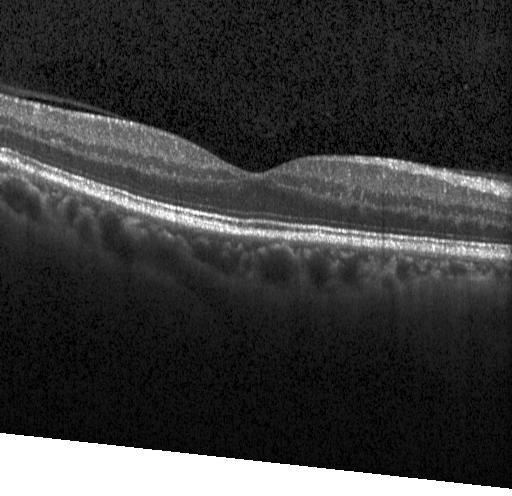
Horizontal scan through the fovea; Heidelberg Spectralis; OCT line scan
Impression: neither choroidal neovascularization, diabetic macular edema, nor drusen.